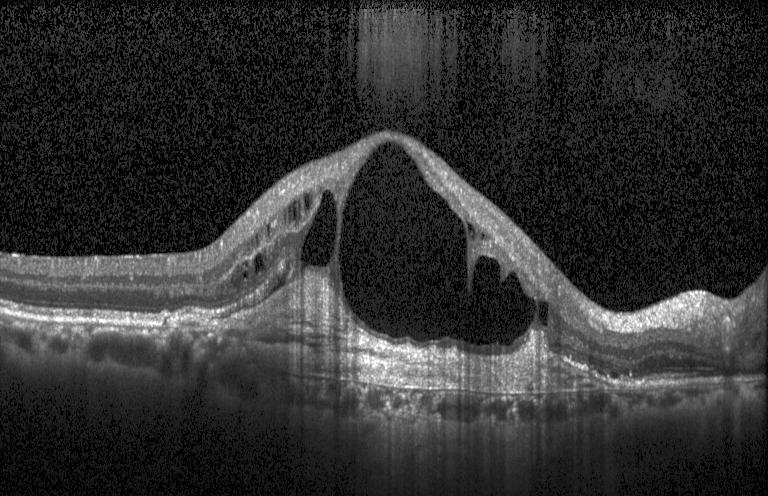

Retinal OCT cross-section
Finding: a choroidal neovascular membrane.